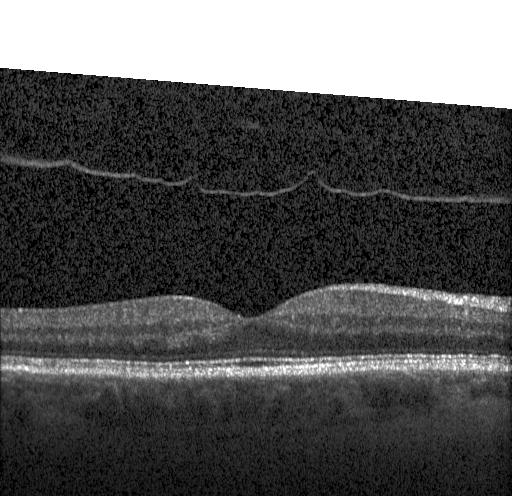
Neither choroidal neovascularization, diabetic macular edema, nor drusen.